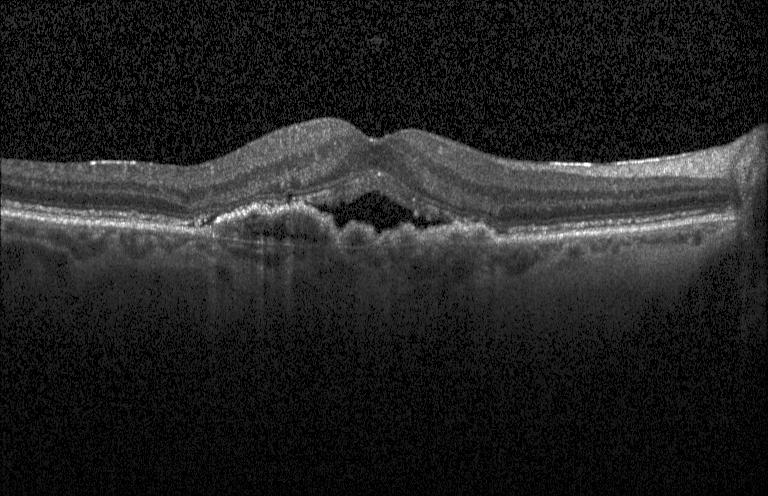 Impression: a choroidal neovascular membrane.